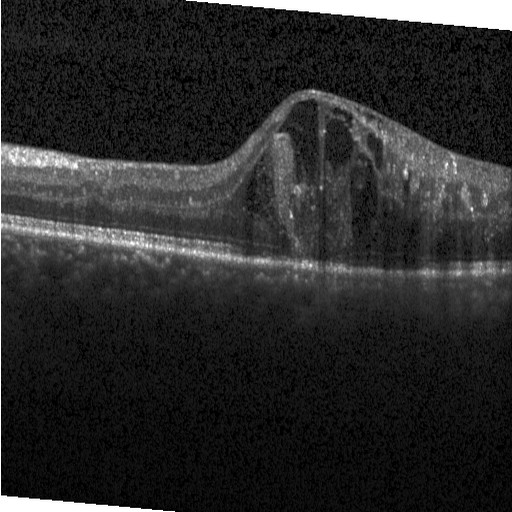 SD-OCT; optical coherence tomography B-scan; through the macula; instrument: Heidelberg Spectralis. Macular OCT: diabetic macular edema.